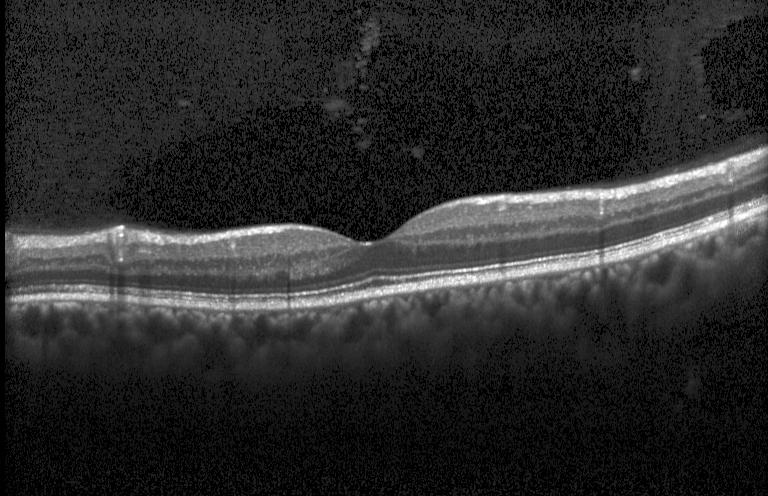 Optical coherence tomography scan. This B-scan demonstrates neither CNV, DME, nor drusen.